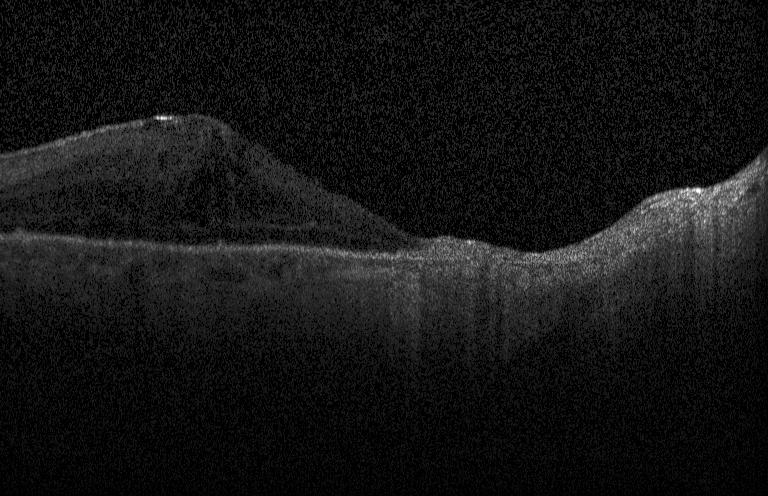
Through the macula. Spectral-domain optical coherence tomography. Optical coherence tomography B-scan — Impression: choroidal neovascularization.